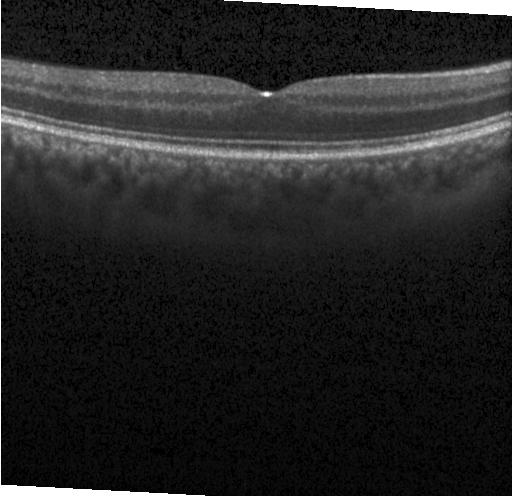

Optical coherence tomography B-scan
Finding: neither choroidal neovascularization, diabetic macular edema, nor drusen.